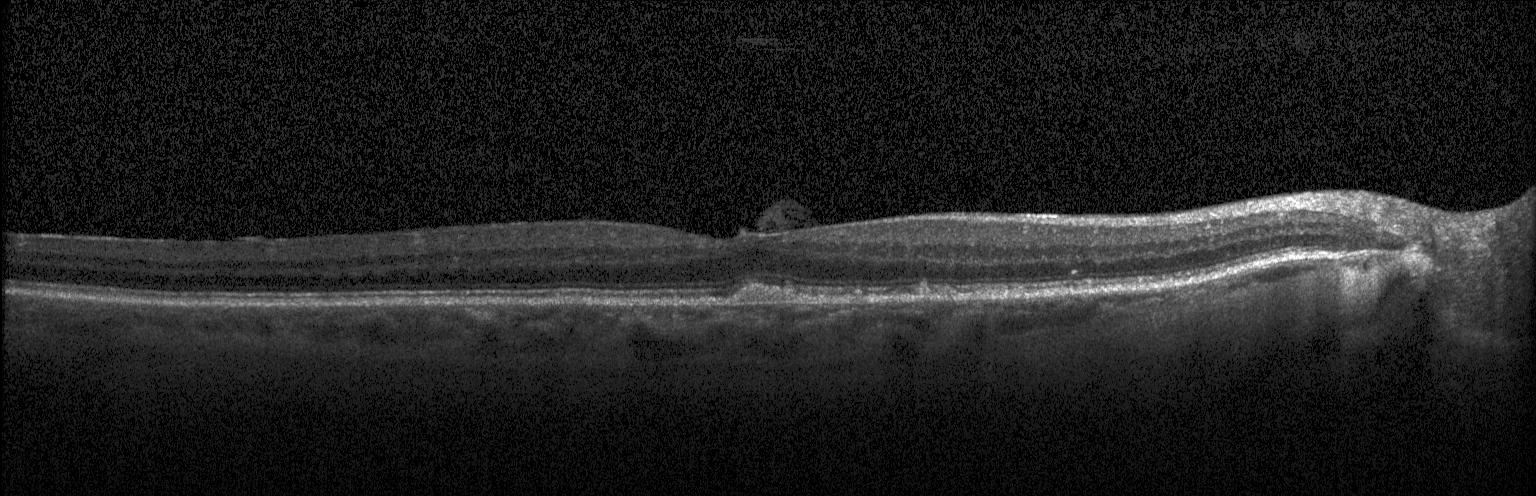 Impression: multiple drusen.